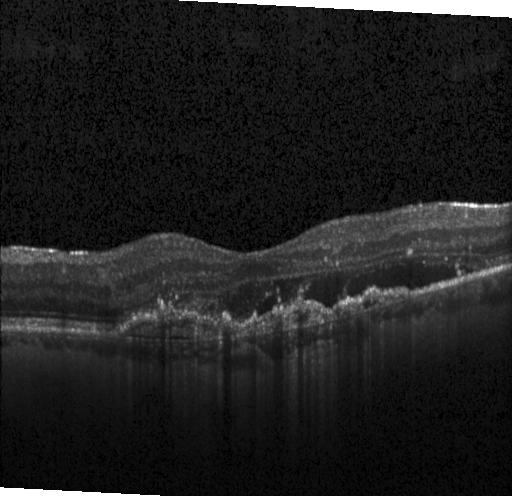 Macular scan · retinal OCT cross-section · acquired on a Heidelberg Spectralis
This B-scan demonstrates a choroidal neovascular membrane.